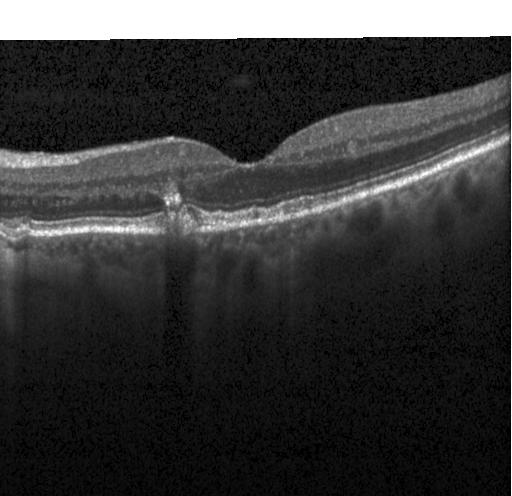 Retinal OCT cross-section. Instrument: Heidelberg Spectralis. Macular scan. Dx: multiple drusen.